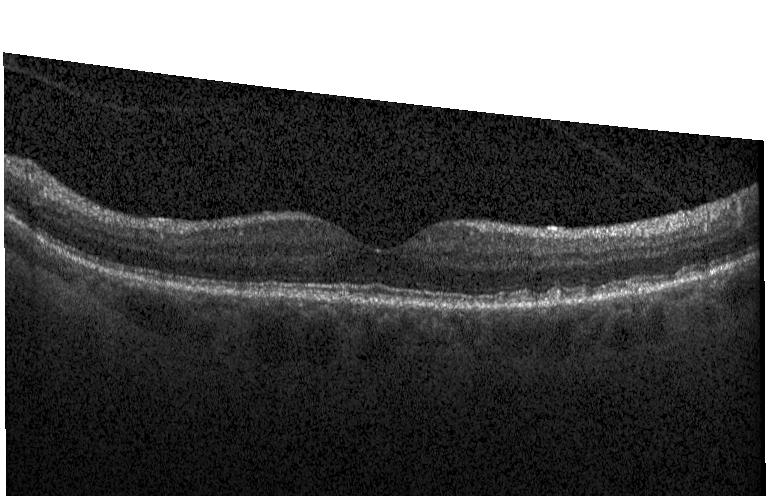 Spectral-domain OCT, through the macula, retinal OCT cross-section, Heidelberg Spectralis. Impression: sub-RPE drusenoid deposits.